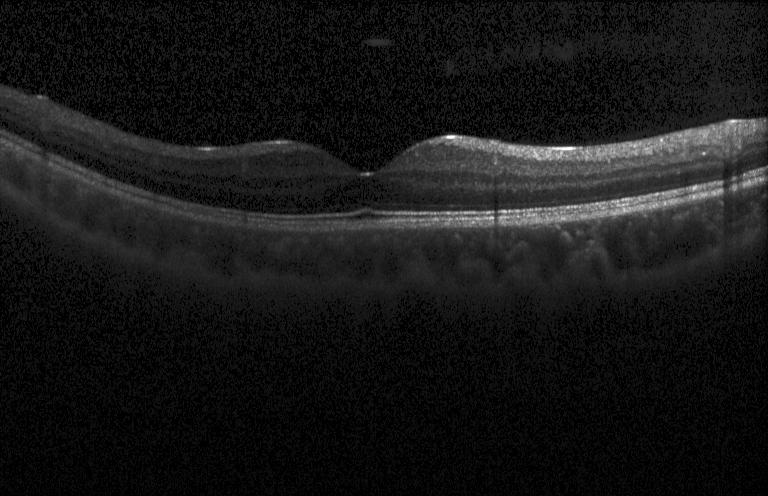

Optical coherence tomography scan · spectral-domain optical coherence tomography · through the macula · acquired on a Heidelberg Spectralis.
Finding: no evidence of choroidal neovascularization, diabetic macular edema, or drusen.